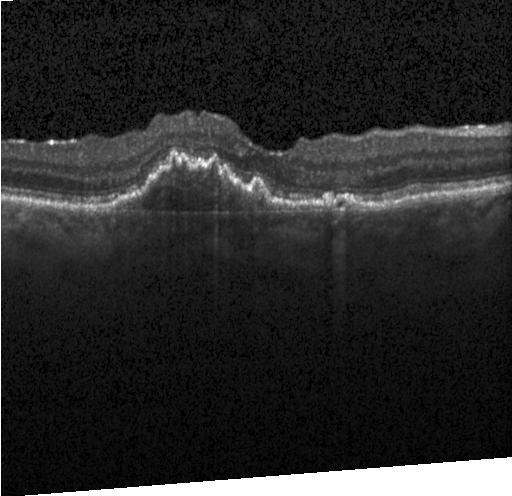

OCT line scan.
Assessment: a choroidal neovascular membrane.